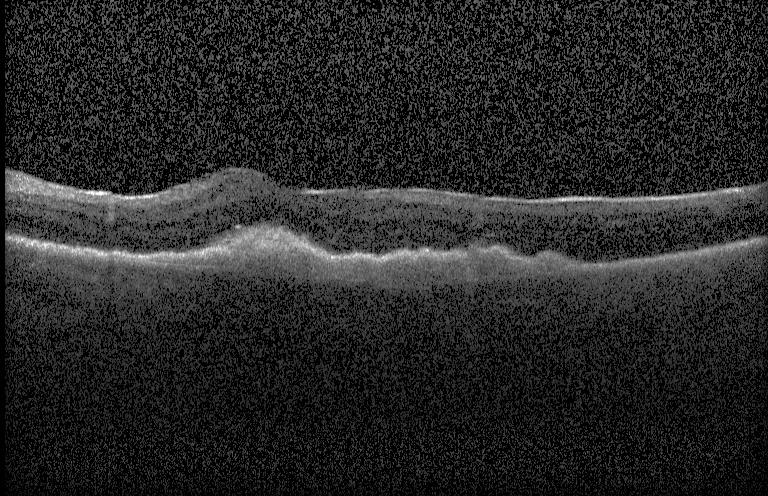 Diagnosis: a choroidal neovascular membrane.